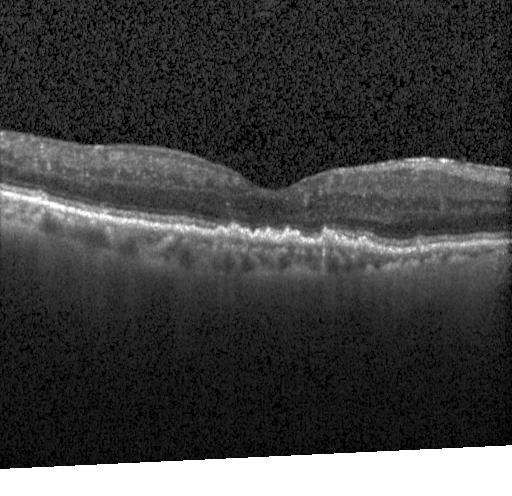

OCT line scan.
Finding: sub-RPE drusenoid deposits.